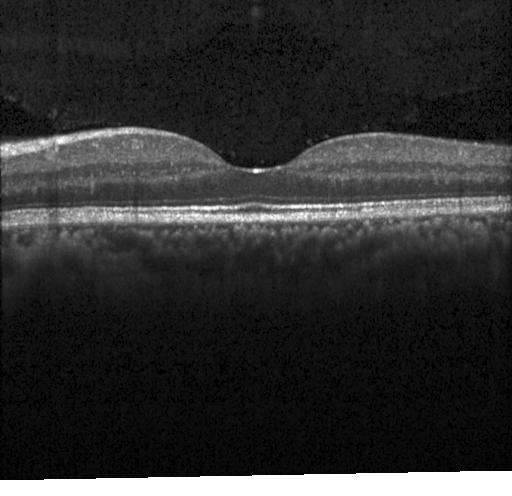
Diagnosis: no evidence of CNV, DME, or drusen.